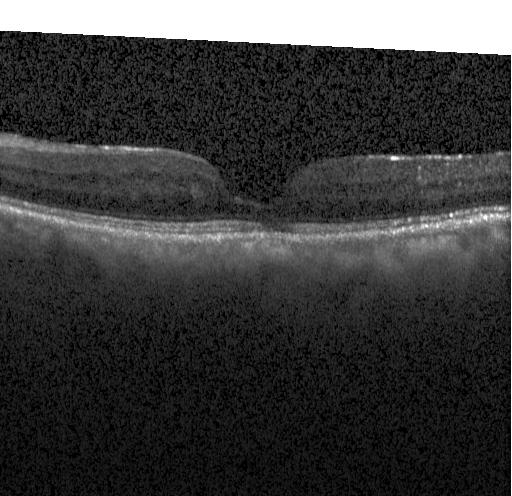 Retinal OCT cross-section — Diagnosis: no evidence of CNV, DME, or drusen.